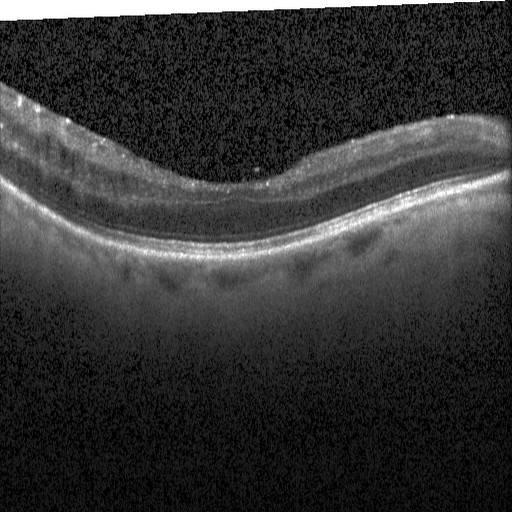
Horizontal scan through the fovea; retinal OCT B-scan; instrument: Heidelberg Spectralis; spectral-domain optical coherence tomography
Finding: DME.